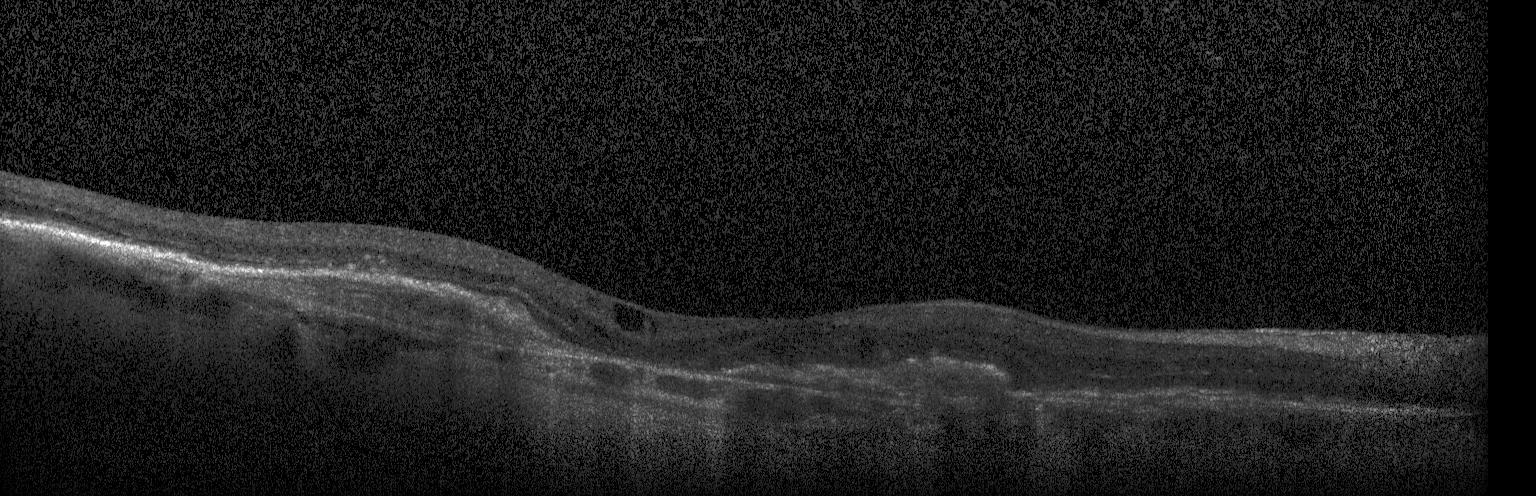
Diagnosis: a choroidal neovascular membrane.